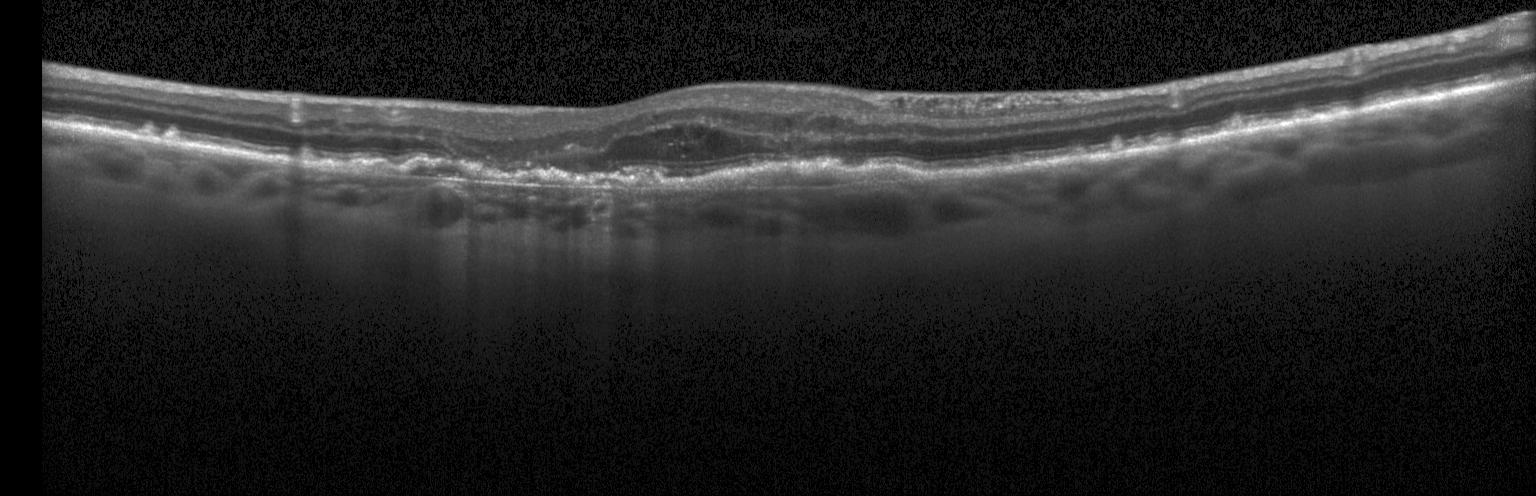
Finding: choroidal neovascularization.